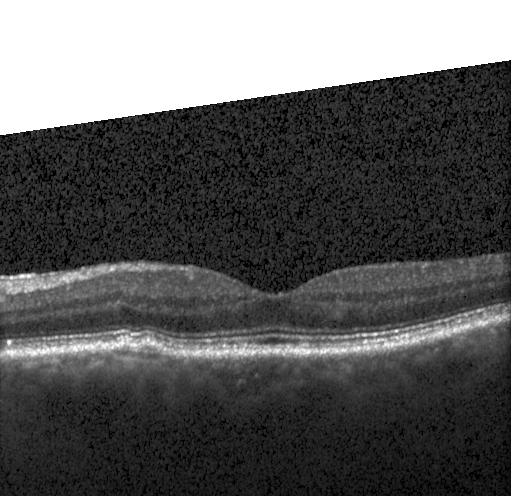 Optical coherence tomography B-scan — Finding: multiple drusen.